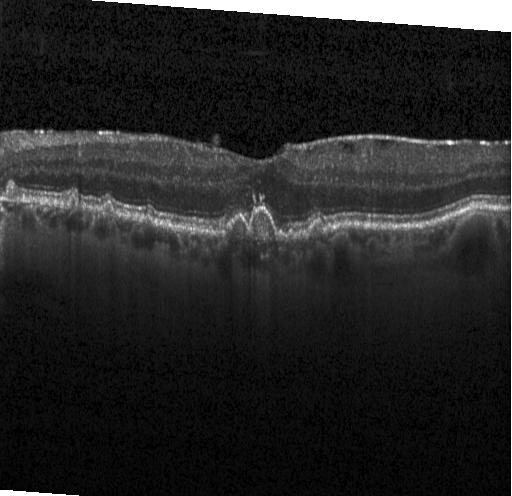 Instrument: Heidelberg Spectralis · SD-OCT · retinal OCT cross-section — Assessment: multiple drusen.